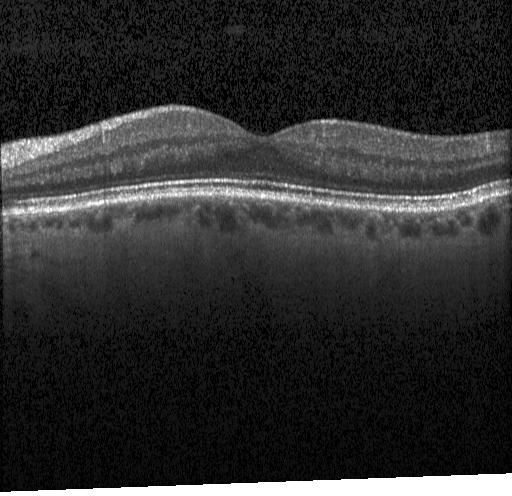

Optical coherence tomography scan.
Assessment: no evidence of choroidal neovascularization, diabetic macular edema, or drusen.